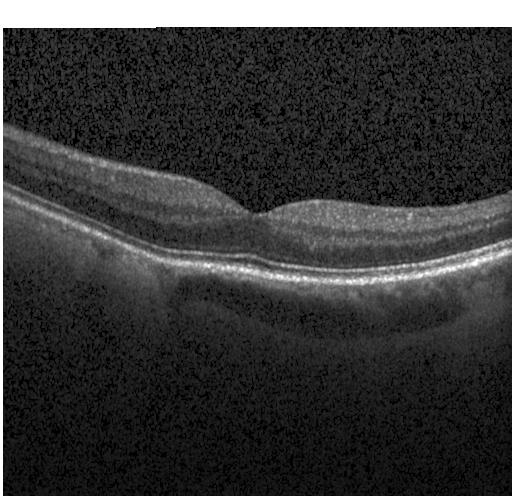

Optical coherence tomography scan; fovea-centered; Heidelberg Spectralis OCT system; SD-OCT — This B-scan demonstrates no evidence of choroidal neovascularization, diabetic macular edema, or drusen.